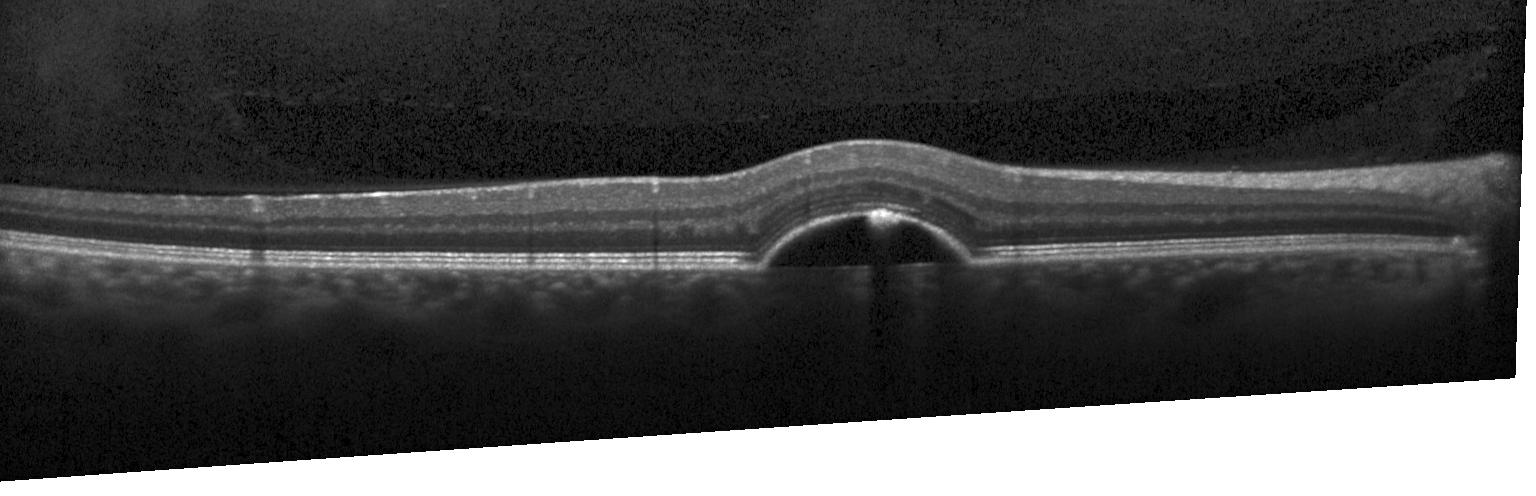

Optical coherence tomography B-scan.
This B-scan demonstrates choroidal neovascularization.